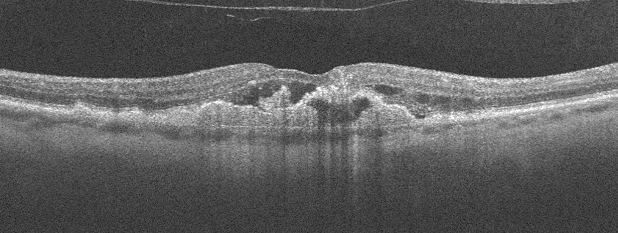

Oculus dexter · retinal OCT B-scan · macular scan · Optovue Avanti RTVue XR — Impression: age-related macular degeneration (AMD).